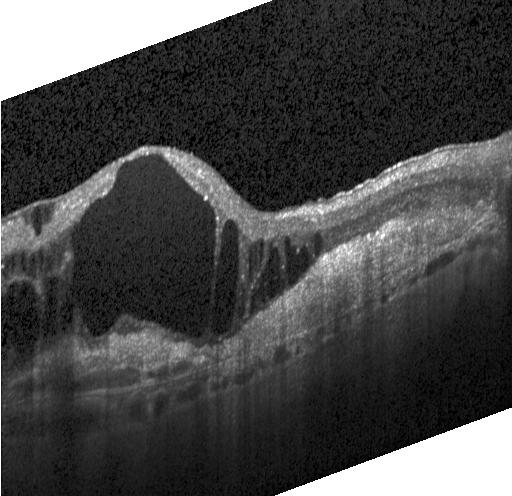 CNV.